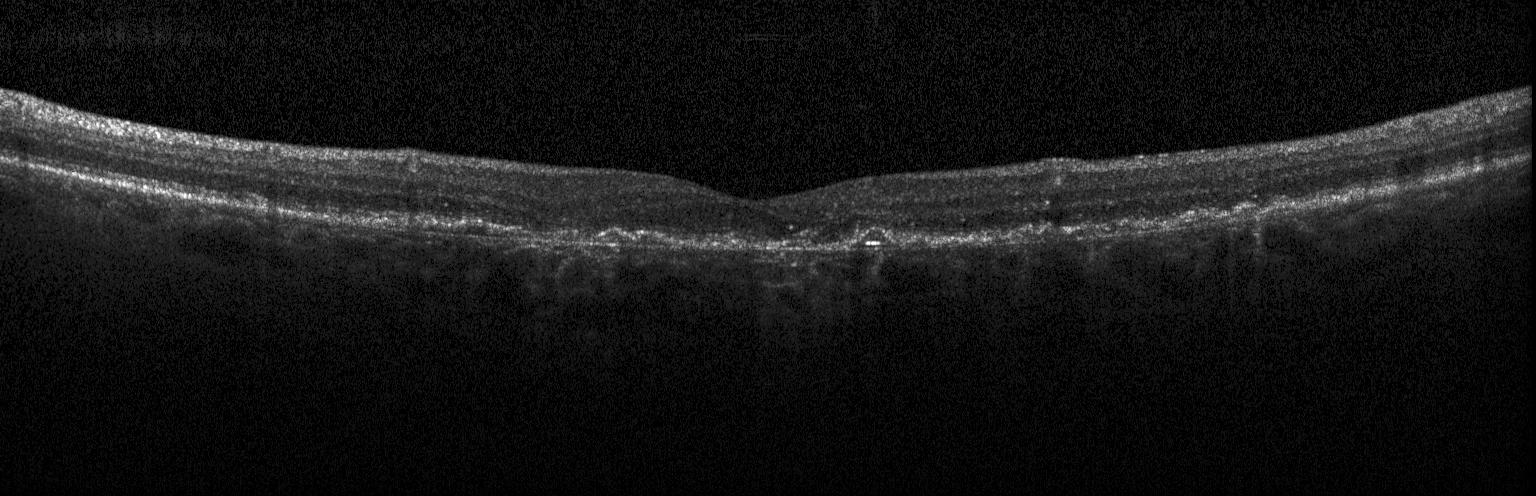

Retinal OCT B-scan. Diagnosis: choroidal neovascularization.